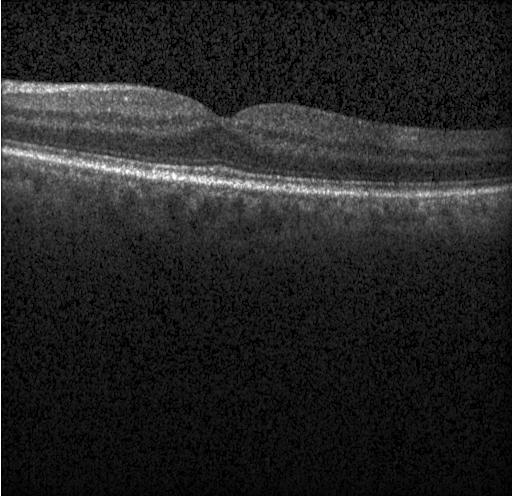
OCT B-scan. No evidence of choroidal neovascularization, diabetic macular edema, or drusen.